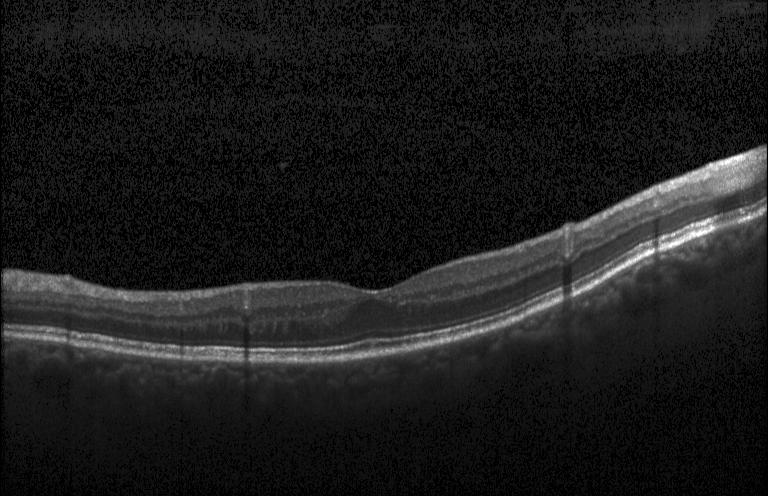

OCT B-scan.
Diagnosis: no choroidal neovascularization, diabetic macular edema, or drusen.